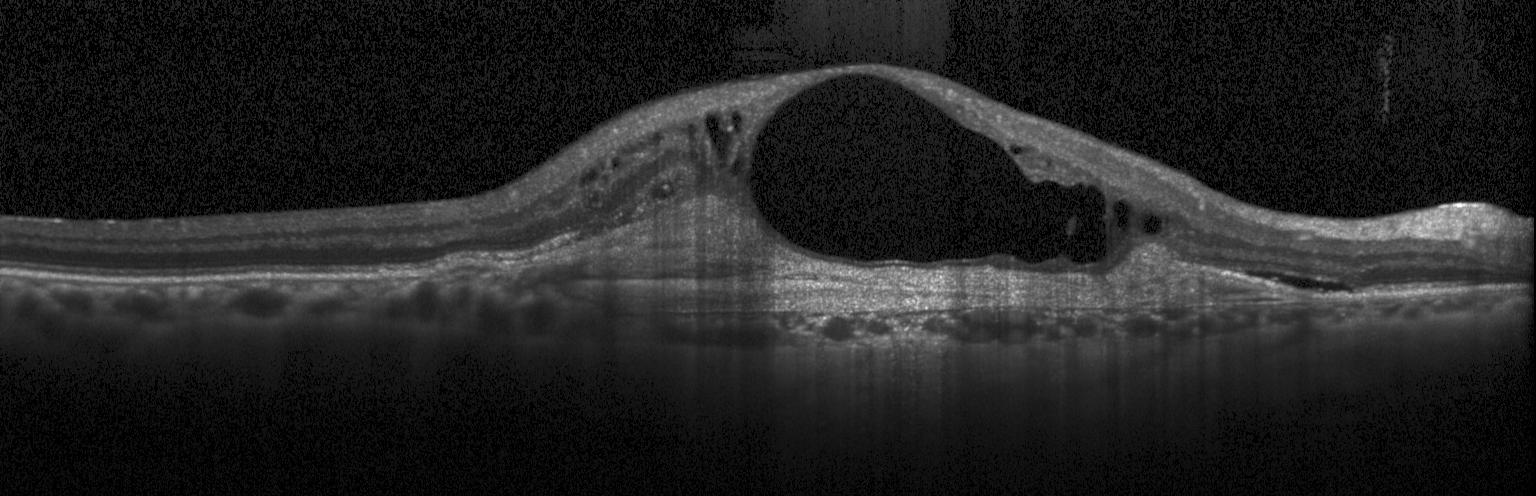
OCT line scan — Diagnosis: choroidal neovascularization.